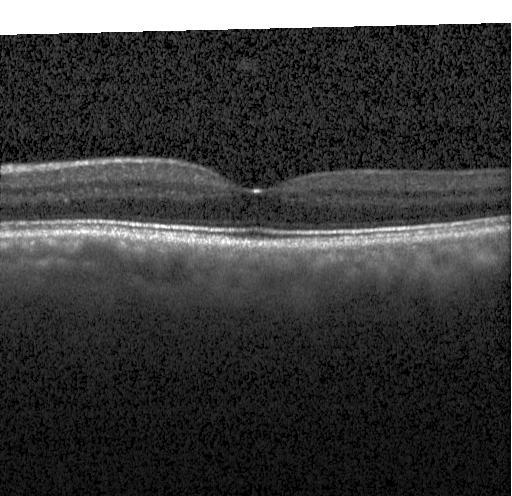
Optical coherence tomography B-scan — Finding: no choroidal neovascularization, diabetic macular edema, or drusen.